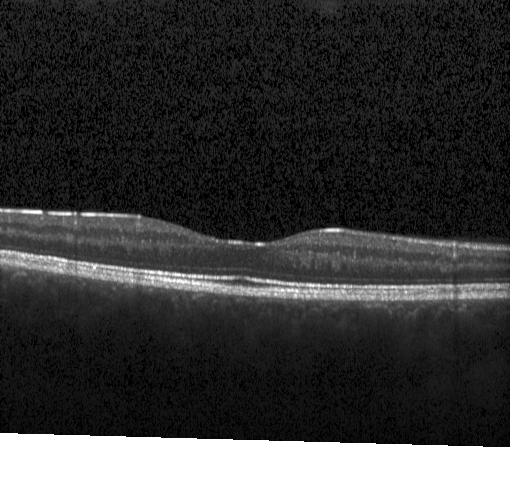 Centered on the fovea, Heidelberg Spectralis OCT system, optical coherence tomography B-scan, spectral-domain optical coherence tomography. No choroidal neovascularization, no diabetic macular edema, and no drusen.